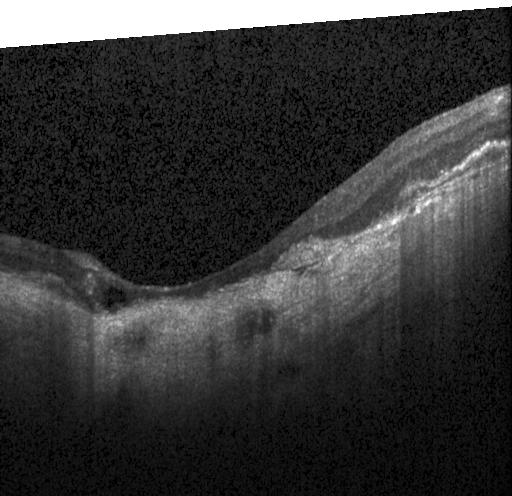

OCT B-scan showing CNV.